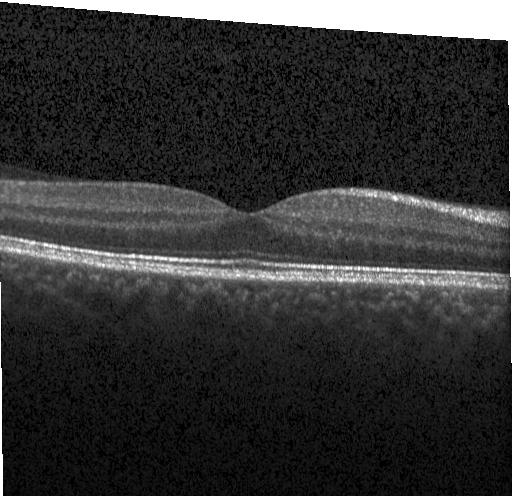
OCT line scan · spectral-domain optical coherence tomography — This B-scan demonstrates no CNV, DME, or drusen.